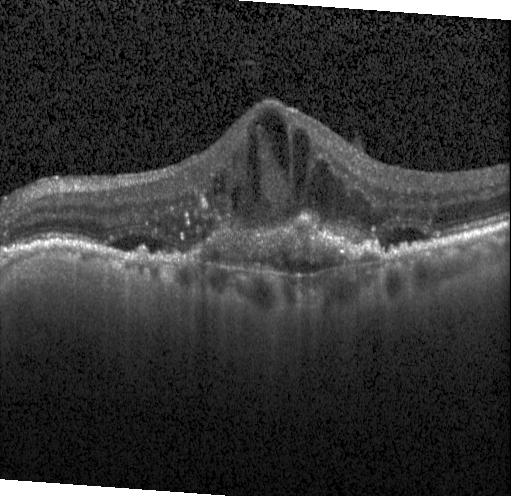

Optical coherence tomography scan.
Diagnosis: a choroidal neovascular membrane.